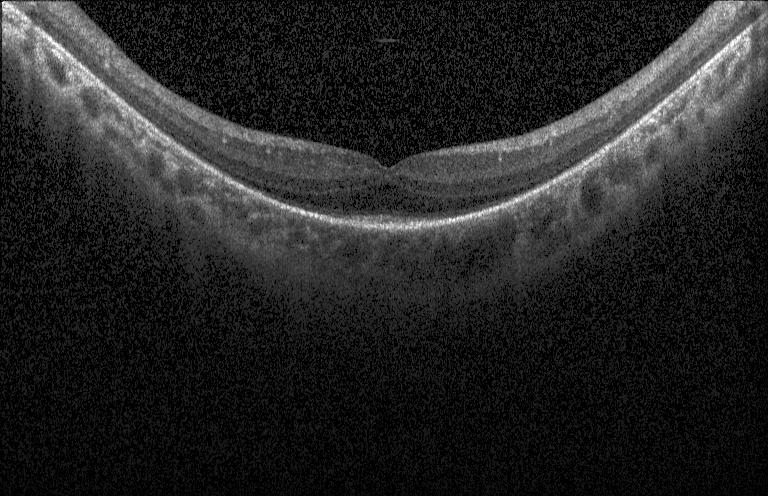 Optical coherence tomography B-scan.
Finding: no CNV, no DME, and no drusen.